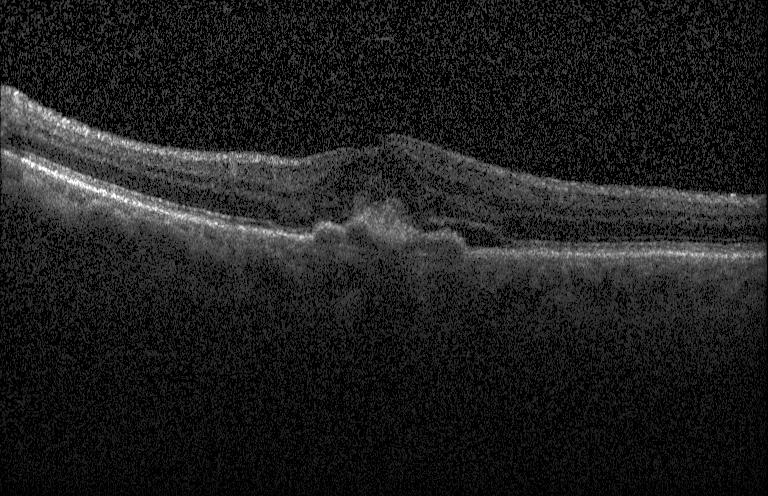
Instrument: Heidelberg Spectralis; centered on the fovea; retinal OCT B-scan.
Assessment: choroidal neovascularization (CNV).